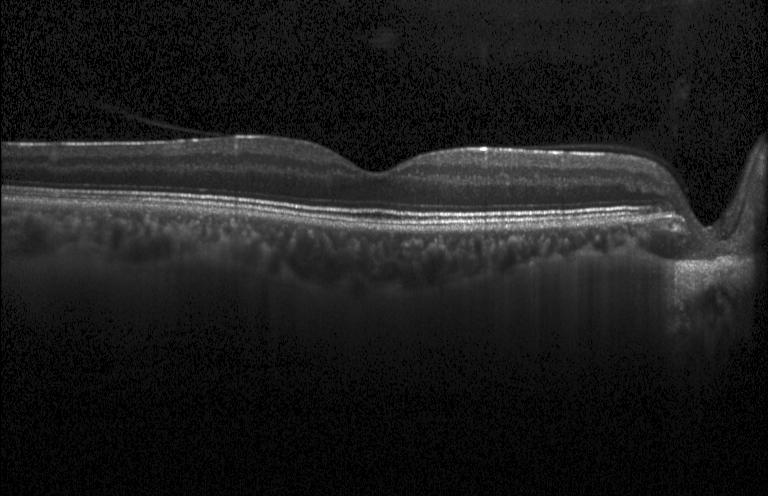

Fovea-centered · OCT B-scan — Diagnosis: neither CNV, DME, nor drusen.